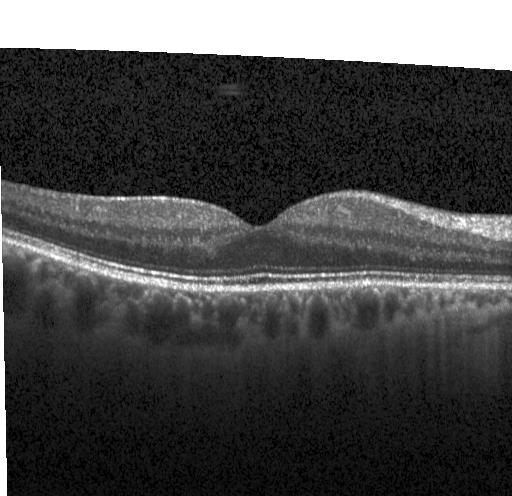
Finding: neither CNV, DME, nor drusen.